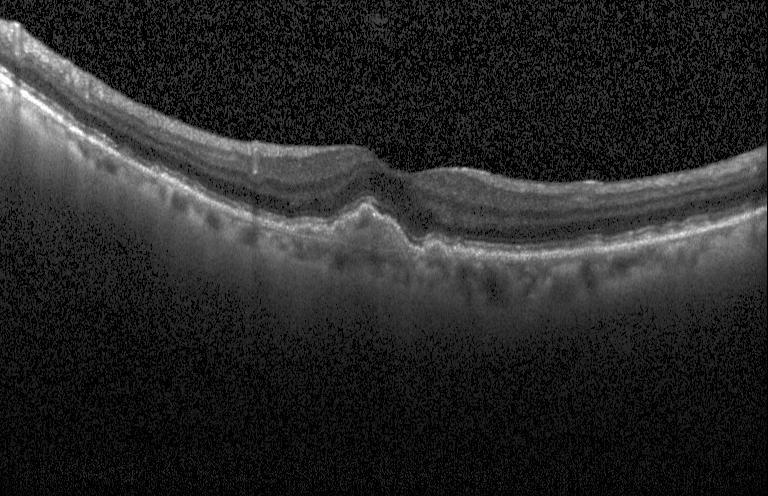 Spectral-domain optical coherence tomography; Heidelberg Spectralis OCT system; optical coherence tomography scan. Finding: a choroidal neovascular membrane.